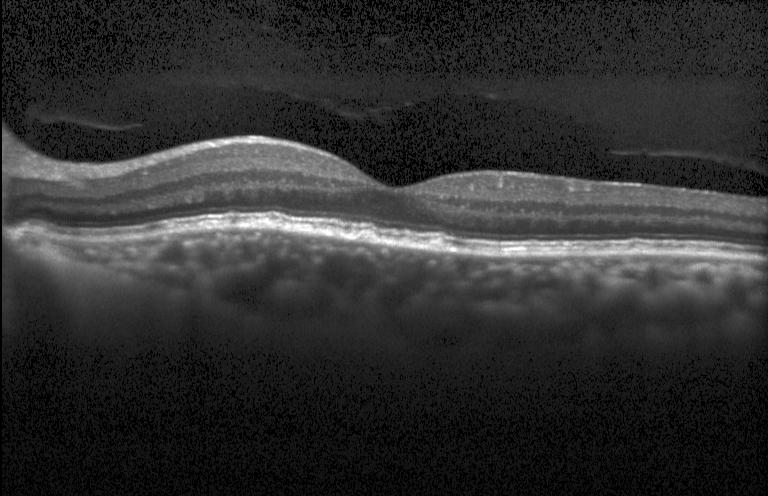

Optical coherence tomography B-scan. Spectral-domain OCT. Heidelberg Spectralis OCT system.
Diagnosis: drusen.